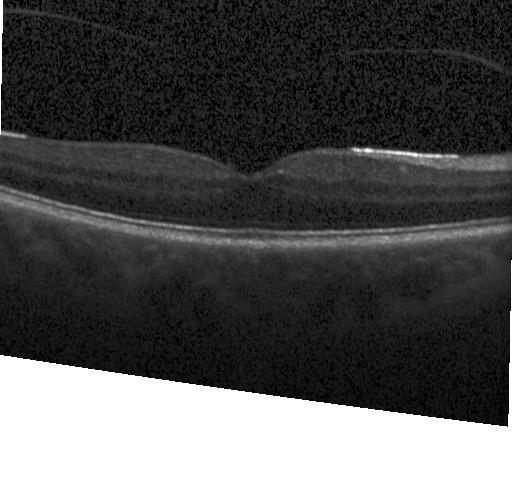 Horizontal scan through the fovea, spectral-domain optical coherence tomography, optical coherence tomography scan
Diagnosis: no evidence of choroidal neovascularization, diabetic macular edema, or drusen.